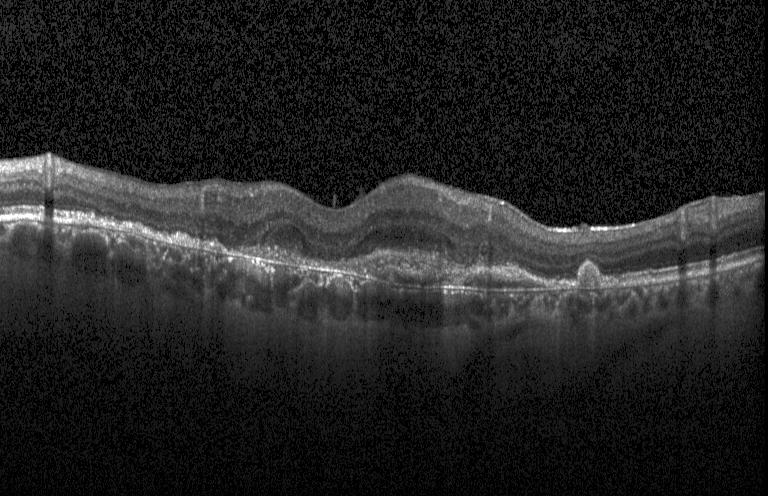

Dx: CNV.